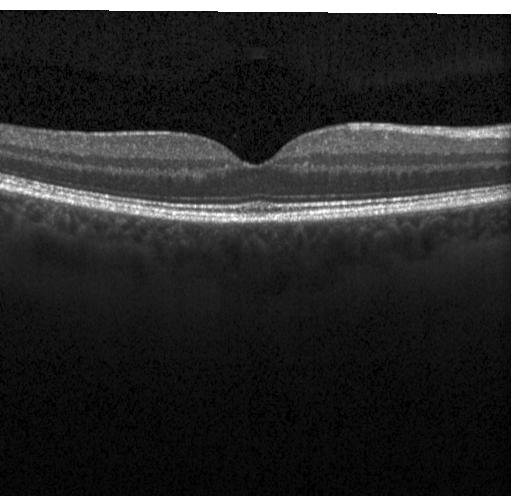
Retinal OCT B-scan.
Dx: no choroidal neovascularization, no diabetic macular edema, and no drusen.